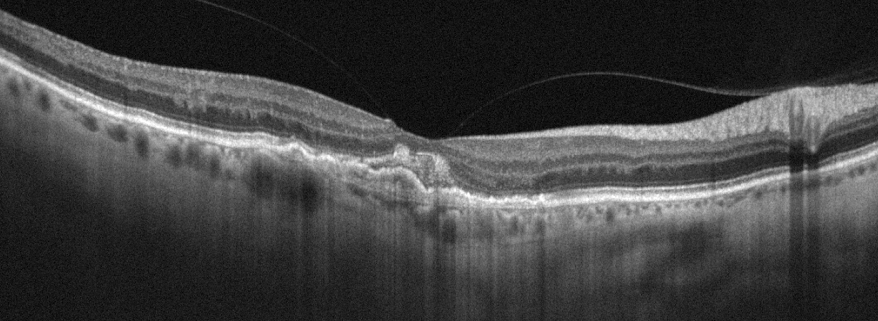 Acquired on an Optovue Avanti RTVue XR, through the macula, optical coherence tomography B-scan.
OCT finding: age-related macular degeneration (AMD).